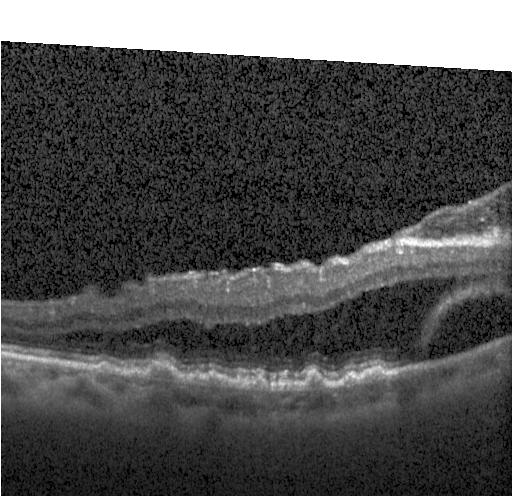

OCT B-scan.
Impression: a choroidal neovascular membrane.